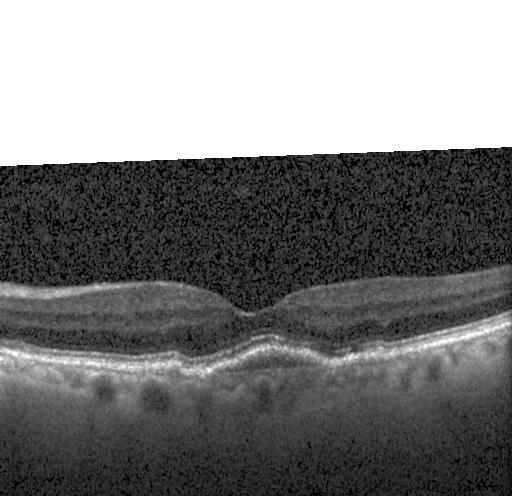 Optical coherence tomography B-scan
Impression: choroidal neovascularization (CNV).